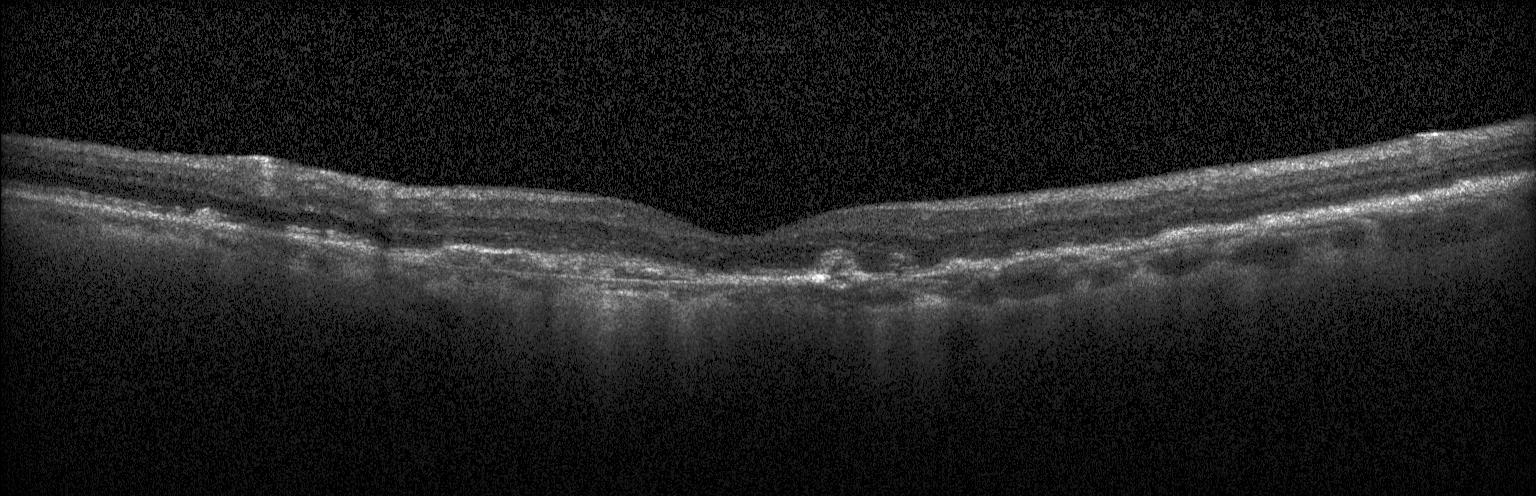

Retinal OCT cross-section showing choroidal neovascularization.